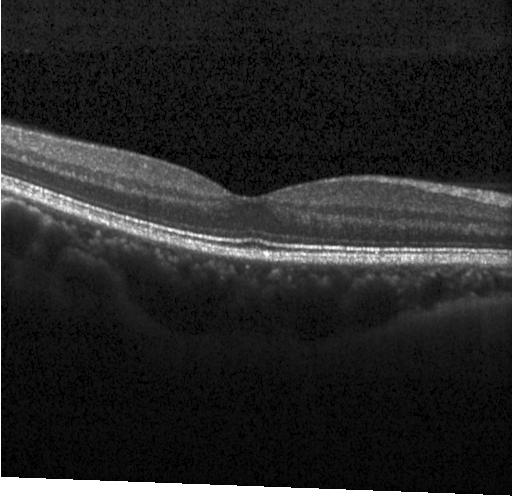

Retinal OCT B-scan. Macular OCT: neither CNV, DME, nor drusen.